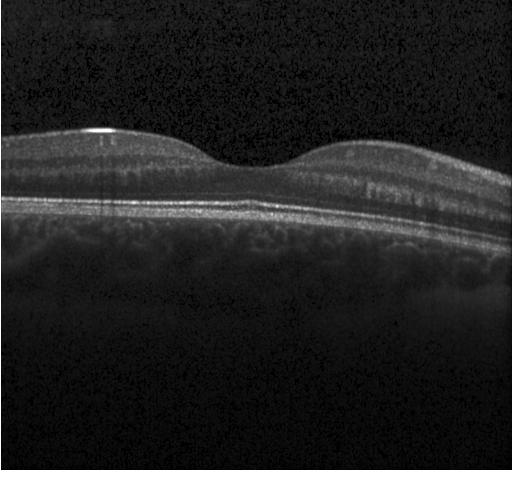
Spectral-domain OCT; centered on the fovea; OCT line scan; acquired on a Heidelberg Spectralis. The scan shows no evidence of choroidal neovascularization, diabetic macular edema, or drusen.